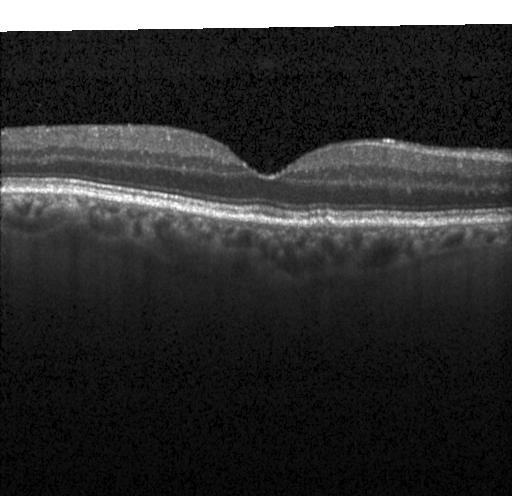

OCT line scan
Diagnosis: sub-RPE drusenoid deposits.